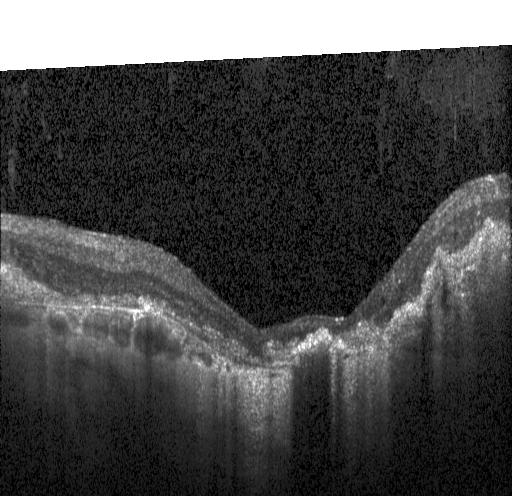 Optical coherence tomography B-scan, spectral-domain OCT, horizontal scan through the fovea — Assessment: a choroidal neovascular membrane.